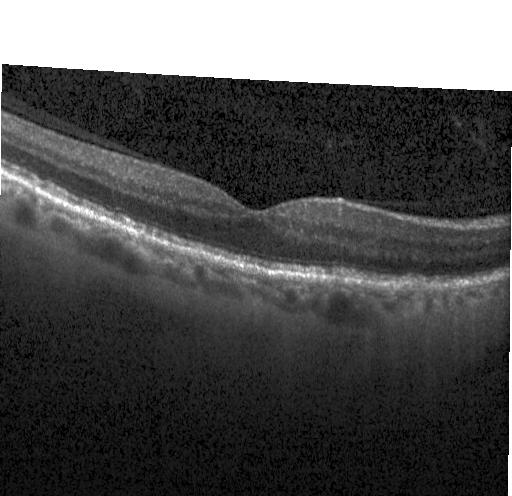
Optical coherence tomography scan; spectral-domain OCT
Dx: no choroidal neovascularization, diabetic macular edema, or drusen.